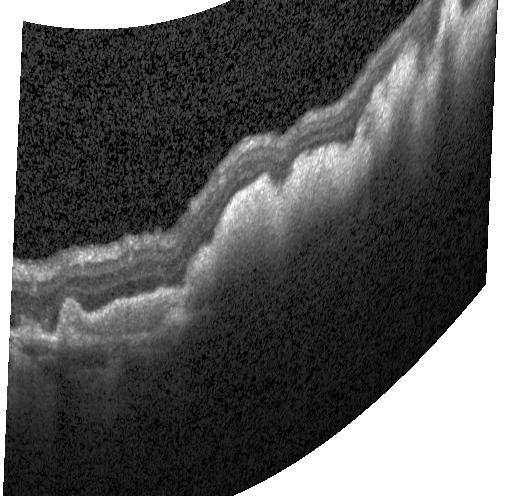
The scan shows choroidal neovascularization.